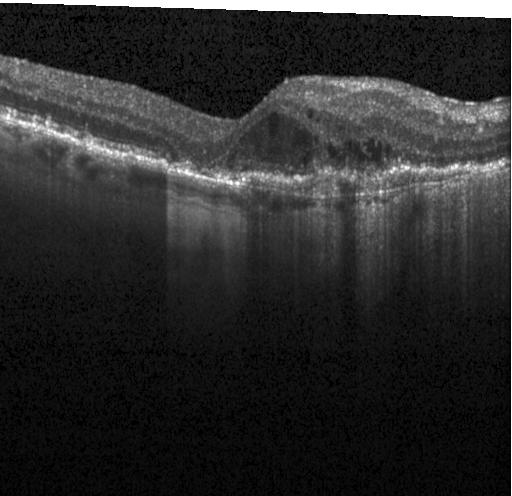
Optical coherence tomography scan, spectral-domain optical coherence tomography
The scan shows a choroidal neovascular membrane.